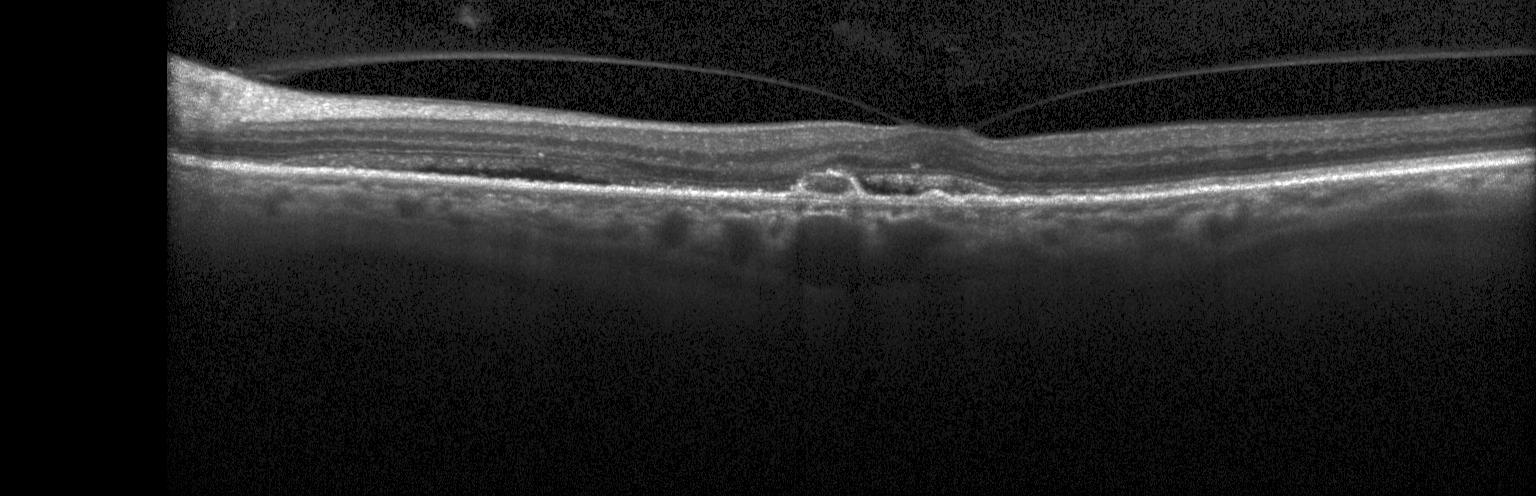
Retinal OCT cross-section, horizontal scan through the fovea, Heidelberg Spectralis OCT system.
Diagnosis: CNV.